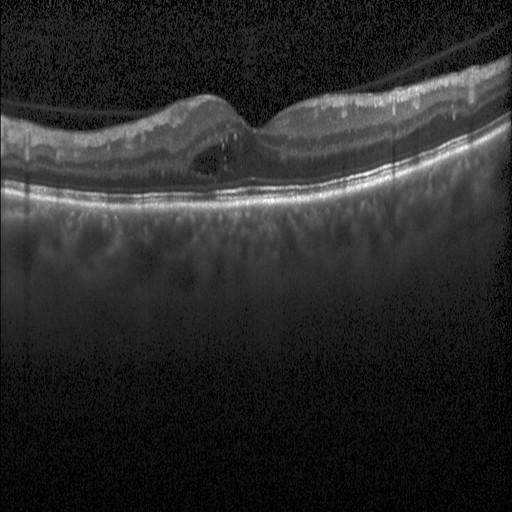 OCT B-scan. Spectral-domain optical coherence tomography.
Impression: diabetic macular edema (DME).